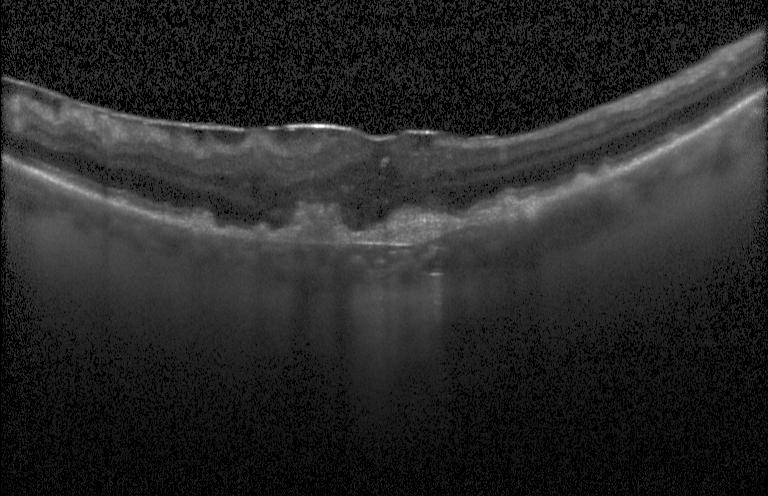

Macular OCT: a choroidal neovascular membrane.